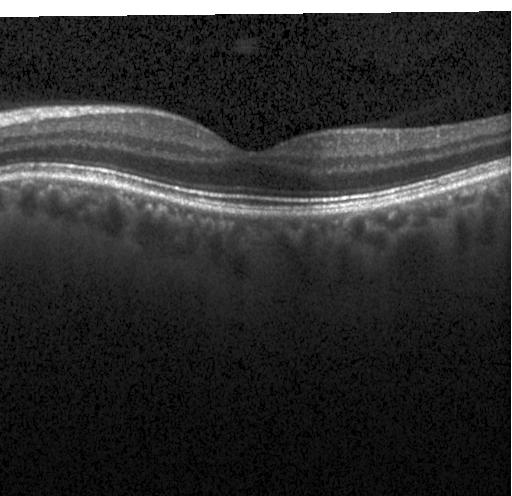

Instrument: Heidelberg Spectralis · spectral-domain OCT · OCT B-scan · macular scan.
Assessment: no choroidal neovascularization, diabetic macular edema, or drusen.